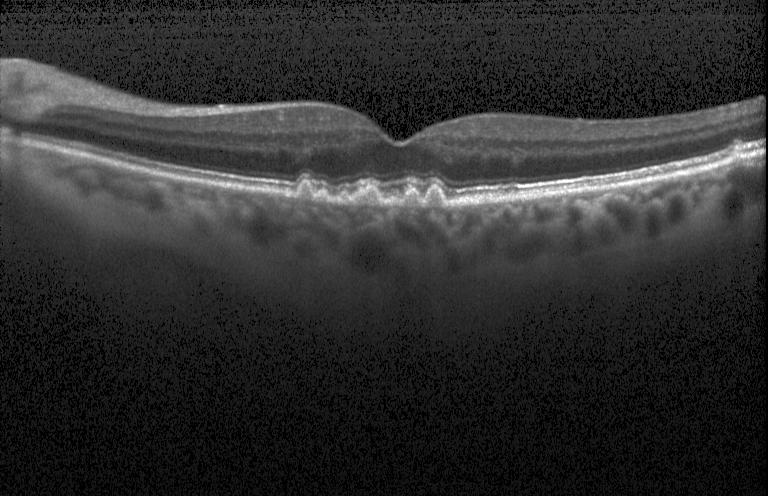

Retinal OCT cross-section. Diagnosis: multiple drusen.